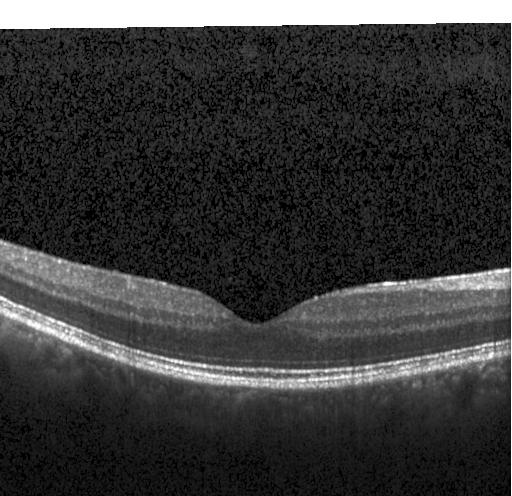
Centered on the fovea; optical coherence tomography B-scan; Heidelberg Spectralis. Finding: neither choroidal neovascularization, diabetic macular edema, nor drusen.